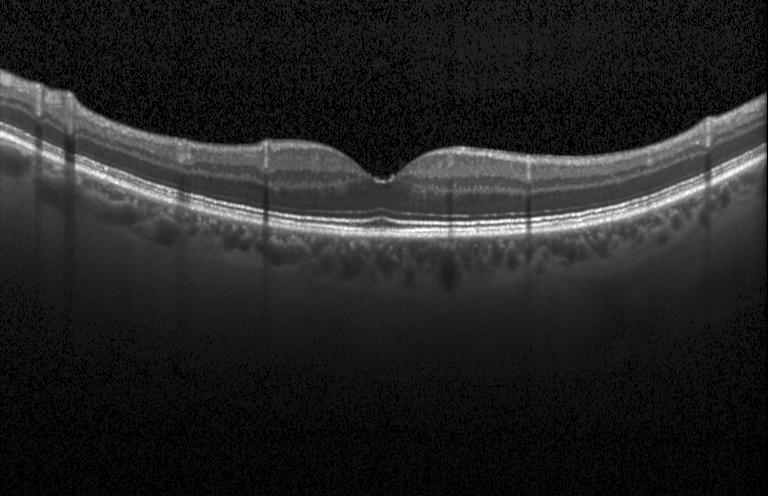
OCT B-scan showing no CNV, no DME, and no drusen.